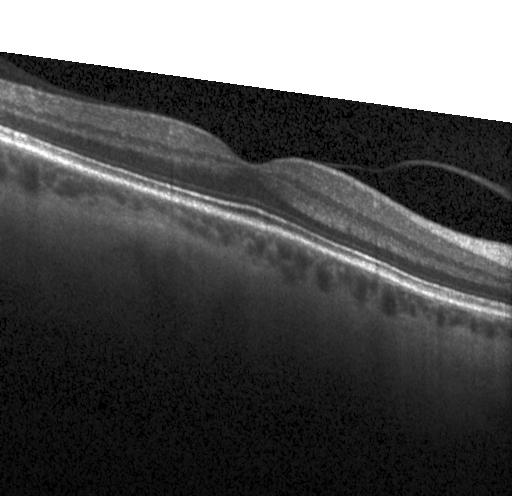

Retinal OCT cross-section. Assessment: neither choroidal neovascularization, diabetic macular edema, nor drusen.